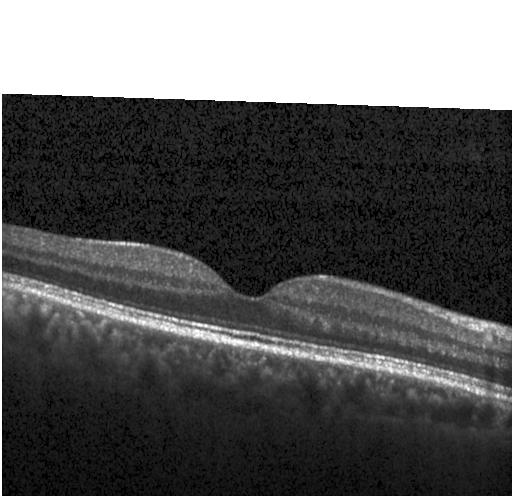 Macular scan · SD-OCT · optical coherence tomography B-scan. OCT finding: no choroidal neovascularization, diabetic macular edema, or drusen.